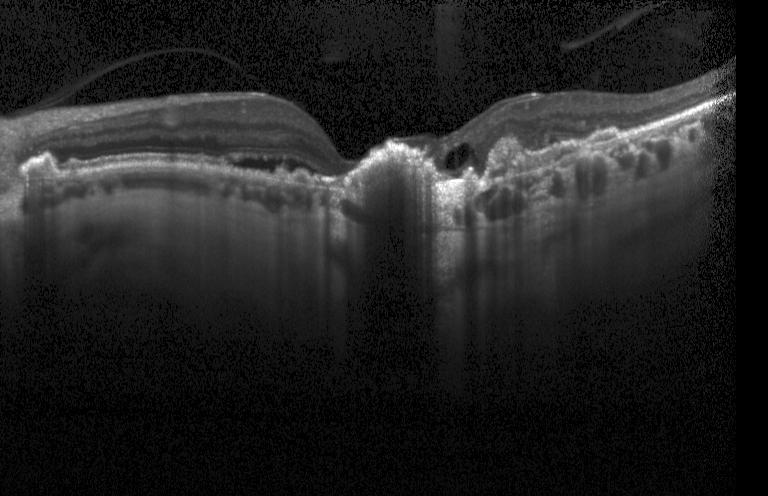 Impression: a choroidal neovascular membrane.